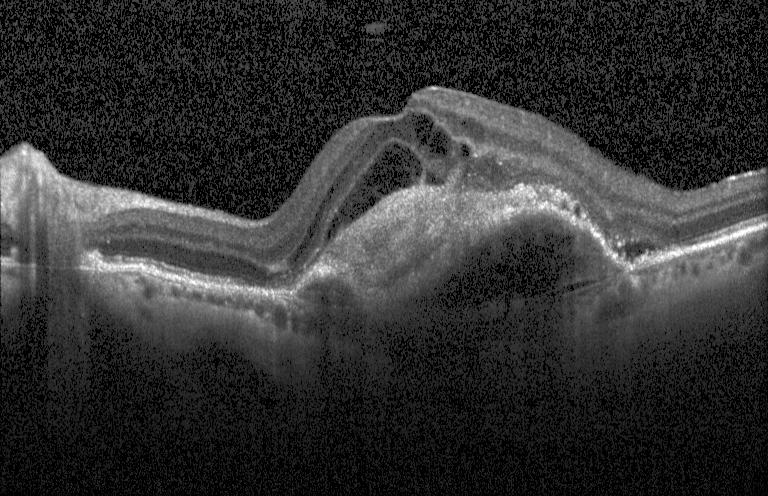

Diagnosis: CNV.